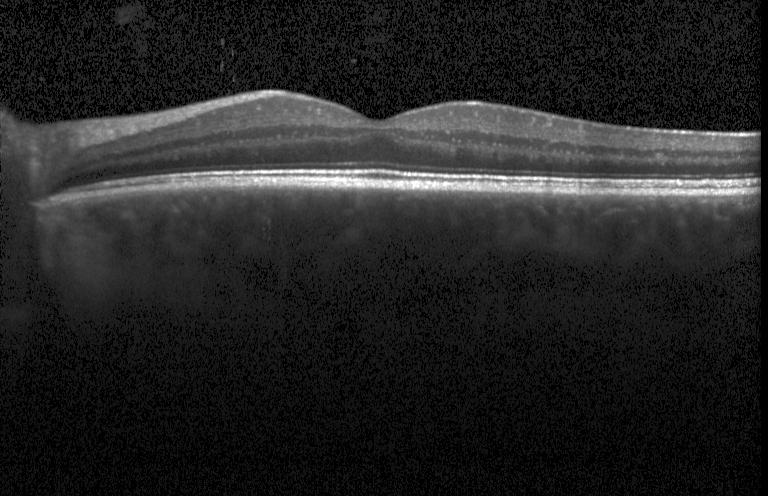 Spectral-domain OCT · optical coherence tomography scan · macular scan — Diagnosis: no choroidal neovascularization, no diabetic macular edema, and no drusen.